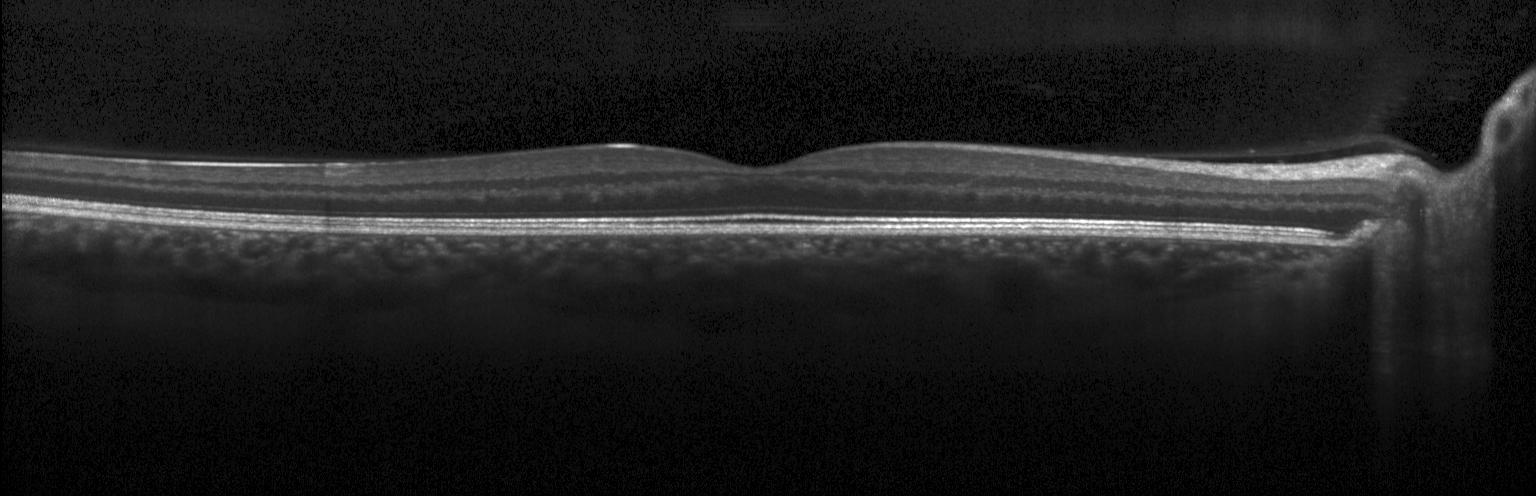 Retinal OCT B-scan, spectral-domain OCT. This B-scan demonstrates no evidence of choroidal neovascularization, diabetic macular edema, or drusen.